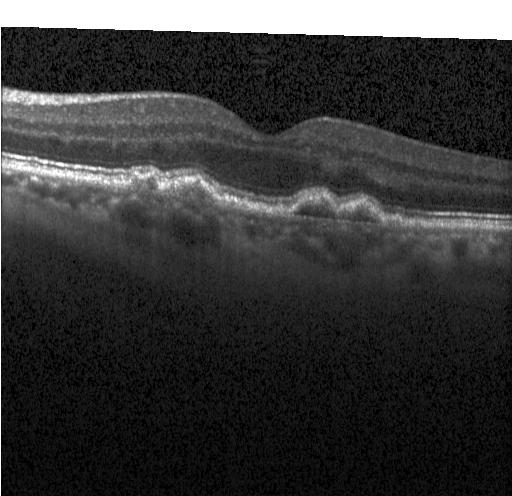

Spectral-domain OCT · OCT line scan · fovea-centered — The scan shows multiple drusen.